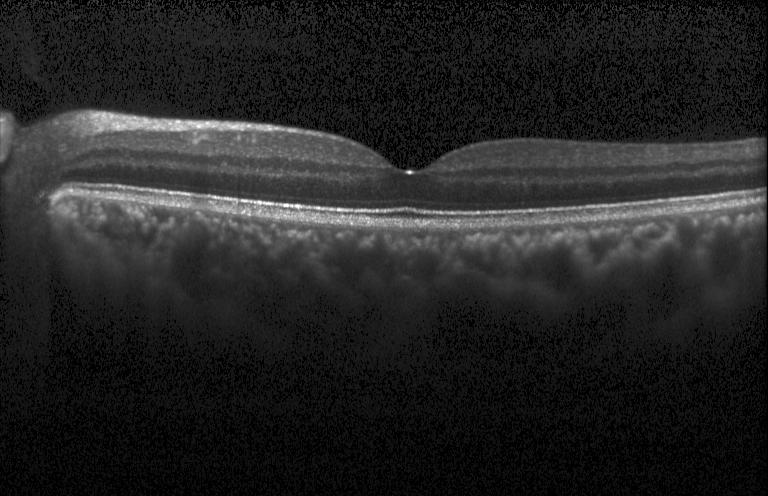 Optical coherence tomography scan · instrument: Heidelberg Spectralis · through the macula — Dx: neither choroidal neovascularization, diabetic macular edema, nor drusen.